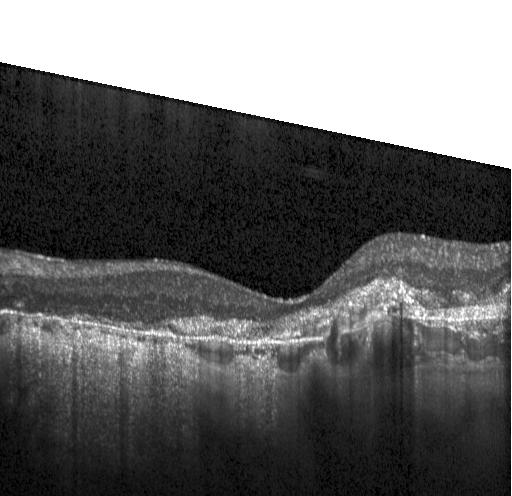

Retinal OCT cross-section showing choroidal neovascularization.